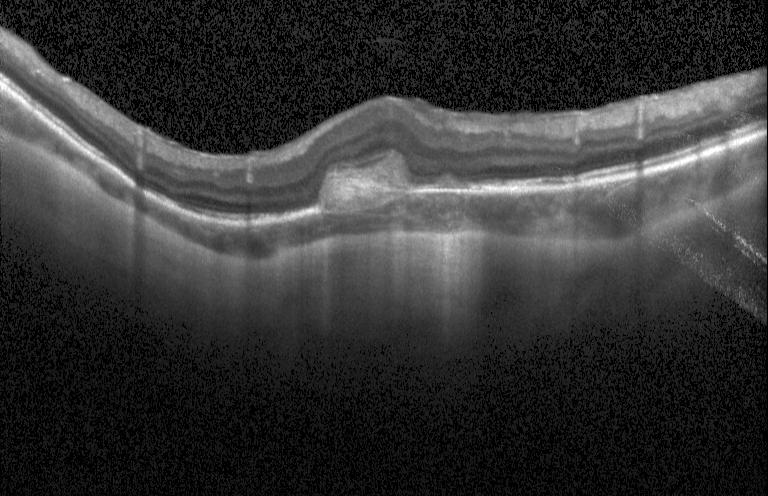
Finding: a choroidal neovascular membrane.